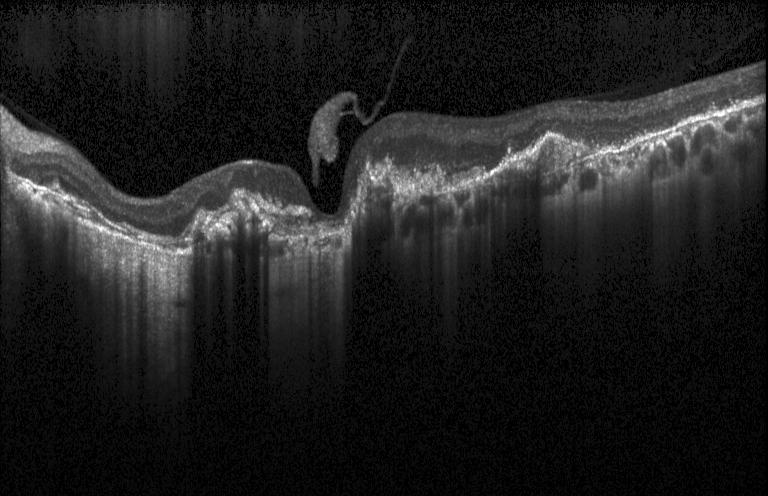
Dx: choroidal neovascularization (CNV).